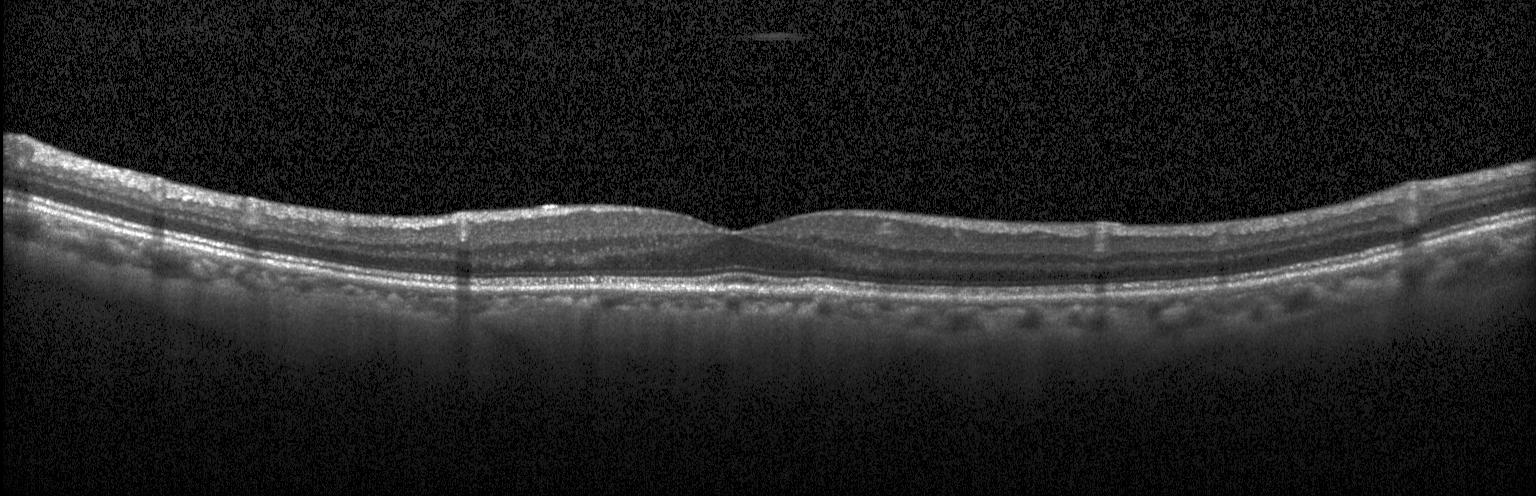 Acquired on a Heidelberg Spectralis; SD-OCT; OCT B-scan — Finding: no choroidal neovascularization, diabetic macular edema, or drusen.